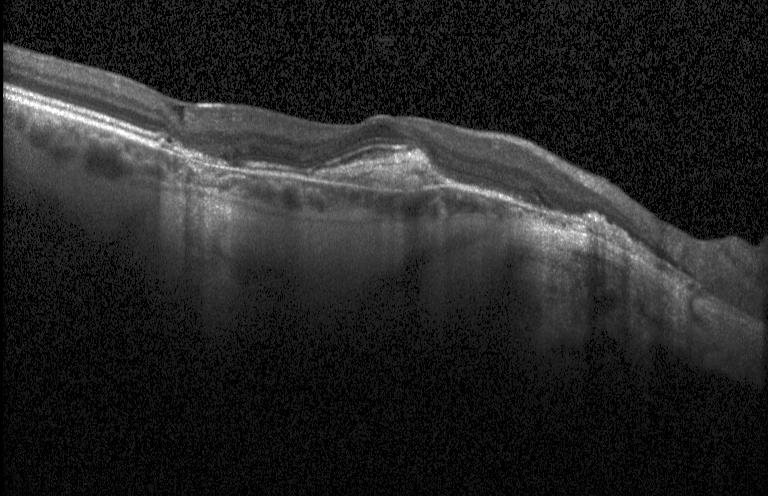
Macular OCT: choroidal neovascularization (CNV).